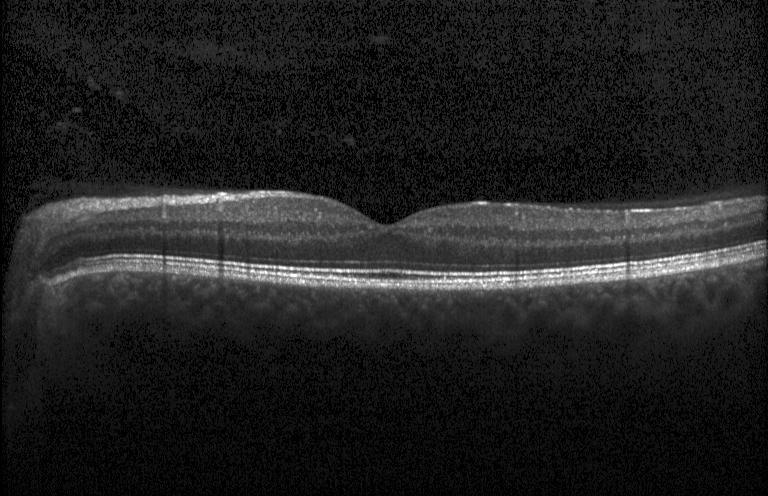

Spectral-domain OCT, optical coherence tomography scan, macular scan. Macular OCT: no evidence of choroidal neovascularization, diabetic macular edema, or drusen.